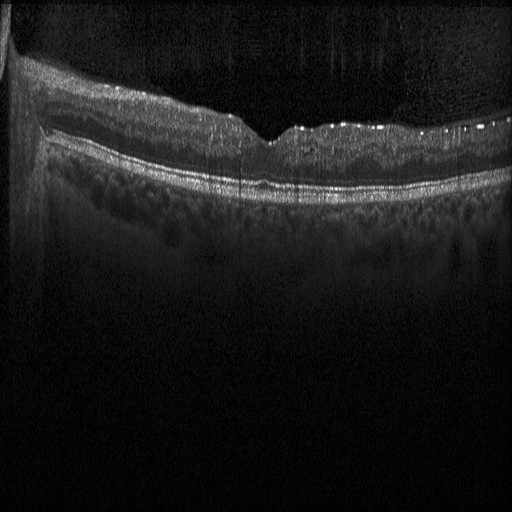 Diagnosis: diabetic macular edema.